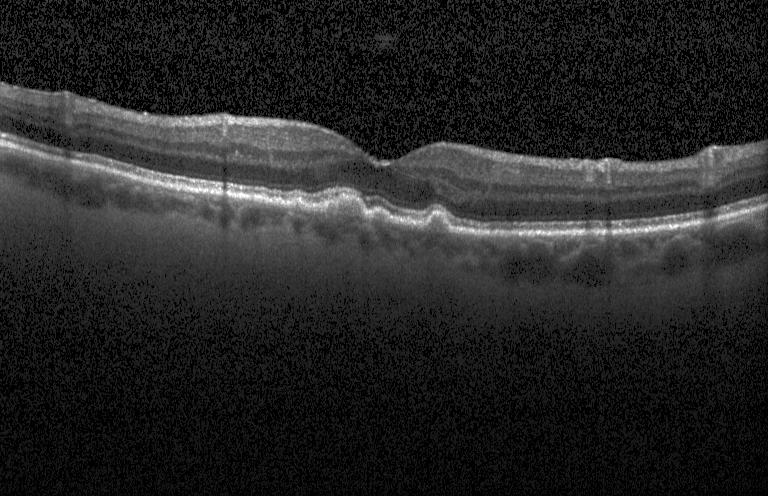

The scan shows drusen.